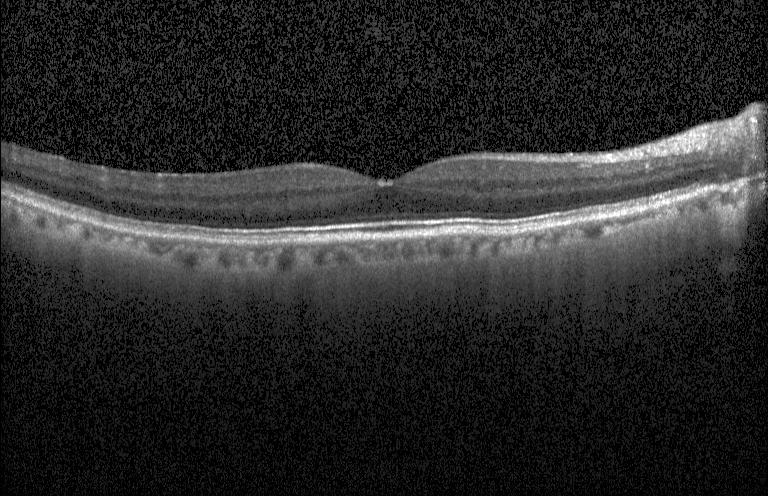
Retinal OCT B-scan · macular scan. Diagnosis: no CNV, no DME, and no drusen.